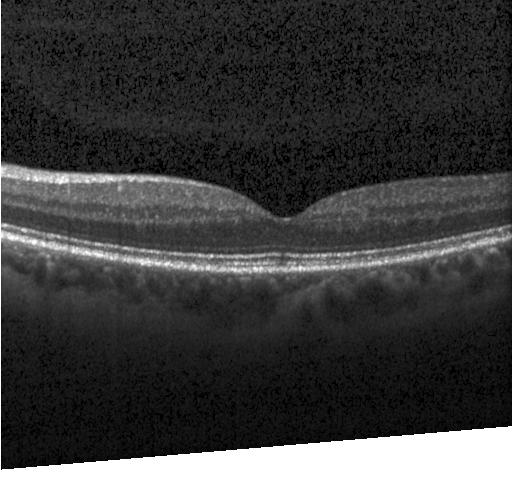
Spectral-domain OCT. OCT B-scan. Horizontal scan through the fovea.
Assessment: no evidence of choroidal neovascularization, diabetic macular edema, or drusen.